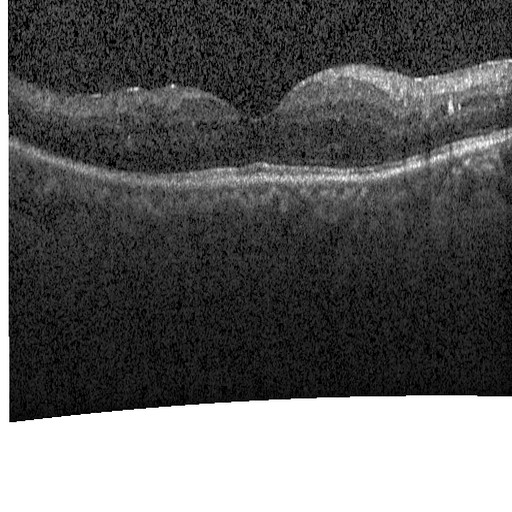

Horizontal scan through the fovea, retinal OCT B-scan. Diabetic macular edema (DME).